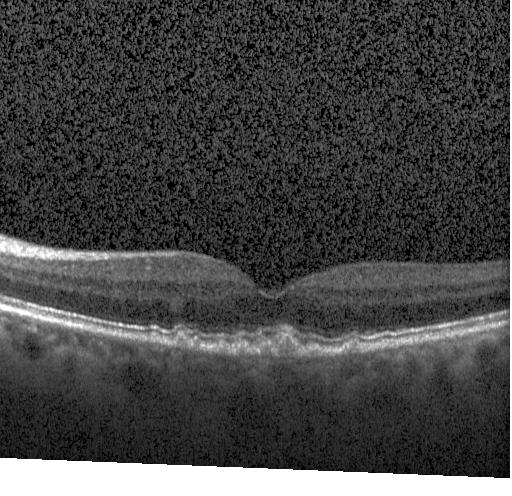

Fovea-centered; optical coherence tomography scan. Finding: multiple drusen.